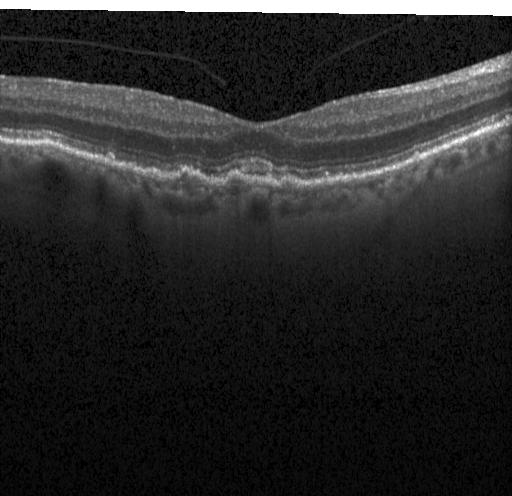

OCT B-scan showing a choroidal neovascular membrane.